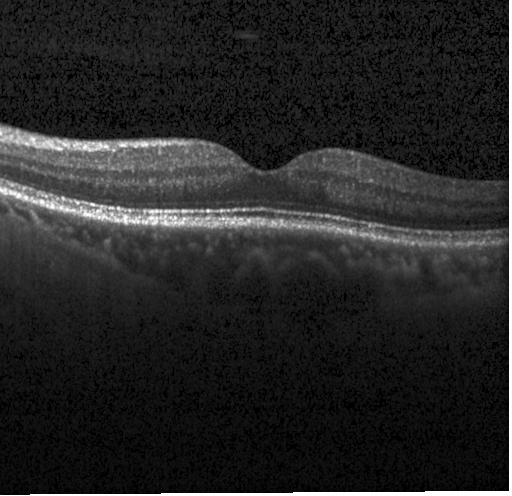

The scan shows no choroidal neovascularization, diabetic macular edema, or drusen.